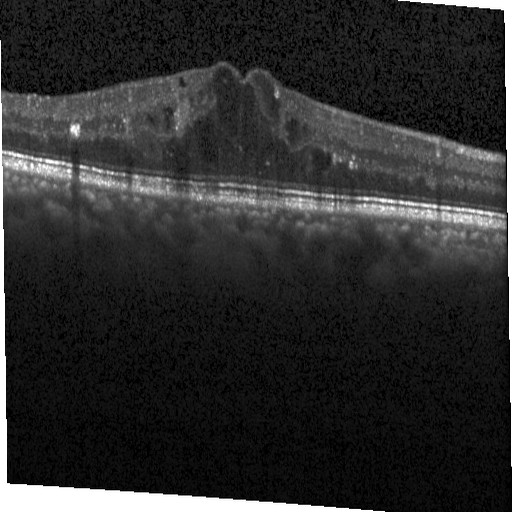
Acquired on a Heidelberg Spectralis; optical coherence tomography scan; SD-OCT
Impression: DME.